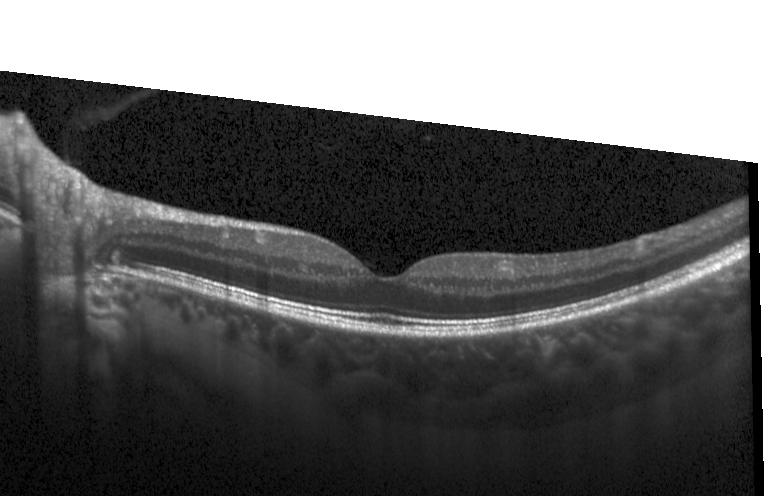 Optical coherence tomography B-scan, fovea-centered. Assessment: neither choroidal neovascularization, diabetic macular edema, nor drusen.